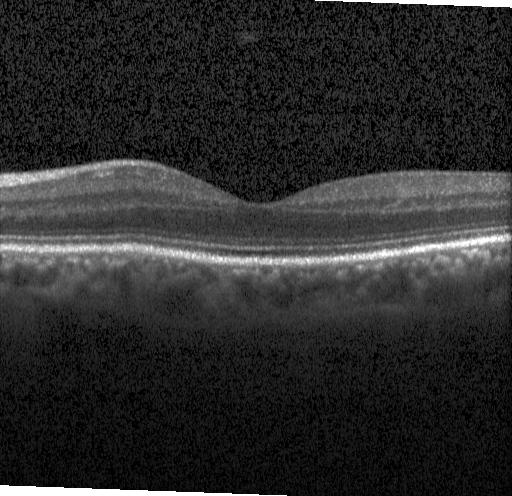

Impression: no choroidal neovascularization, diabetic macular edema, or drusen.